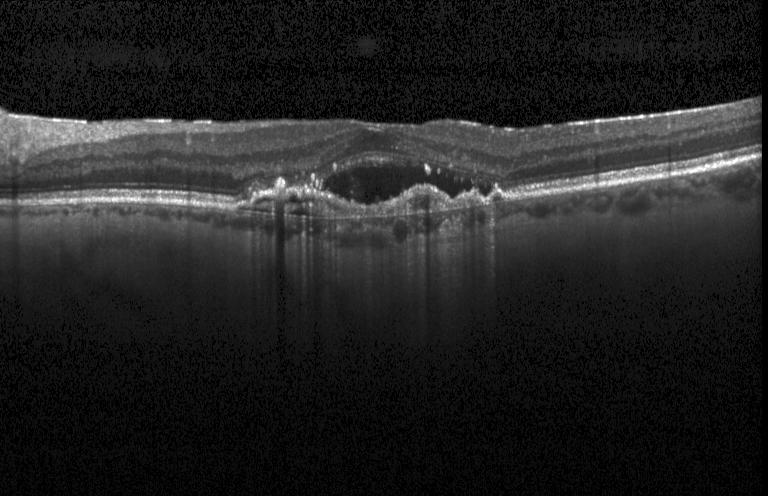

Impression: a choroidal neovascular membrane.